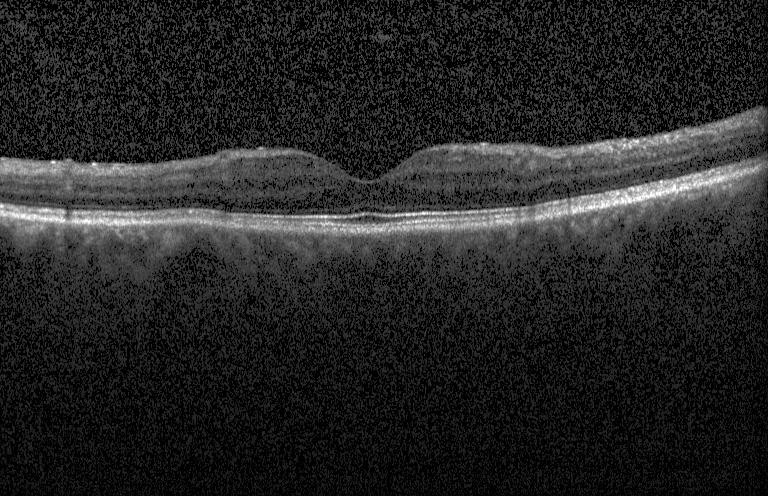 Acquired on a Heidelberg Spectralis. Spectral-domain OCT. OCT B-scan
The scan shows no choroidal neovascularization, diabetic macular edema, or drusen.